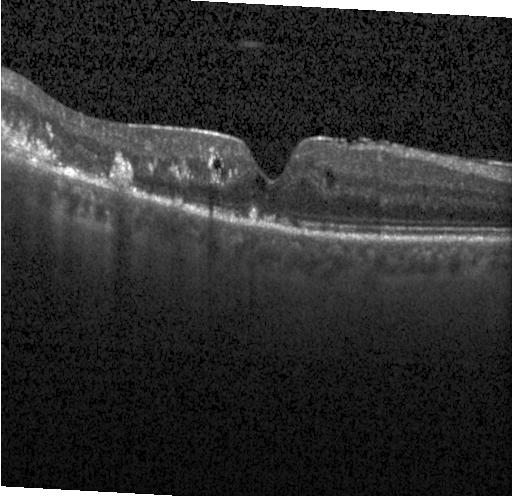

Horizontal scan through the fovea; acquired on a Heidelberg Spectralis; OCT B-scan
Macular OCT: a choroidal neovascular membrane.